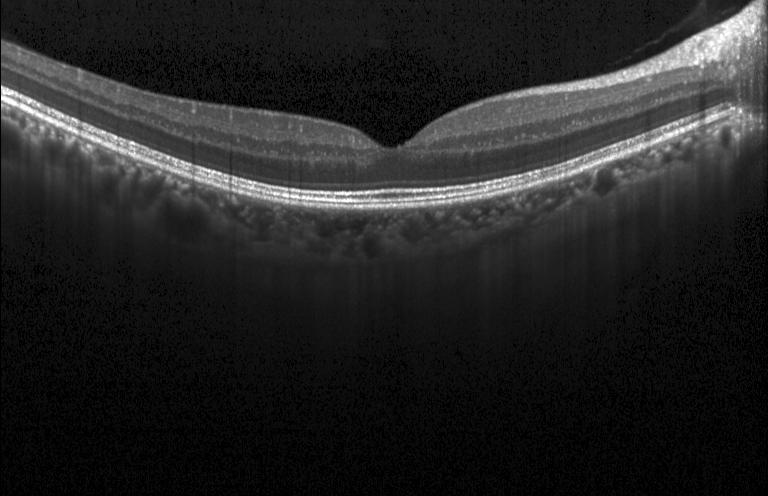

Spectral-domain OCT; acquired on a Heidelberg Spectralis; optical coherence tomography scan; macular scan. The scan shows no choroidal neovascularization, diabetic macular edema, or drusen.